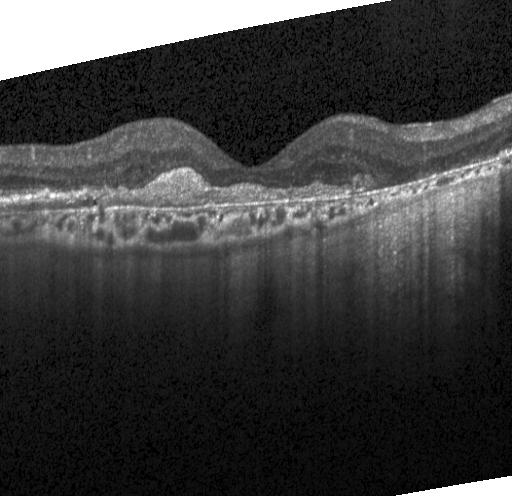

Retinal OCT cross-section showing CNV.